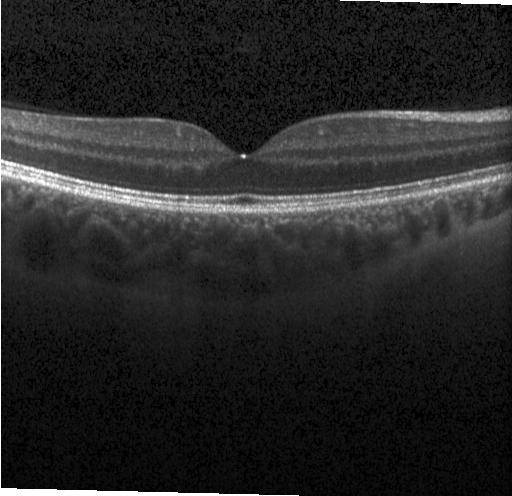 Macular OCT: no evidence of choroidal neovascularization, diabetic macular edema, or drusen.